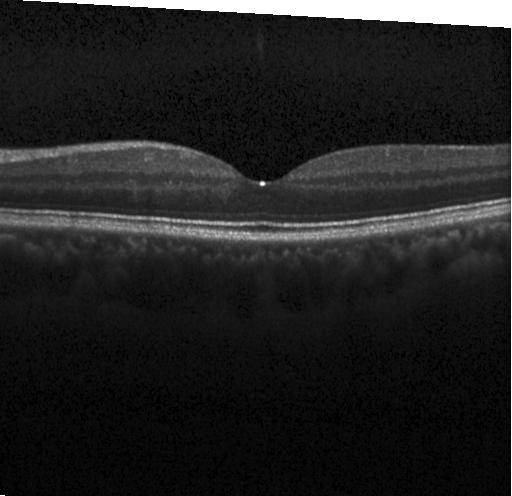 Optical coherence tomography B-scan; fovea-centered — This B-scan demonstrates neither choroidal neovascularization, diabetic macular edema, nor drusen.